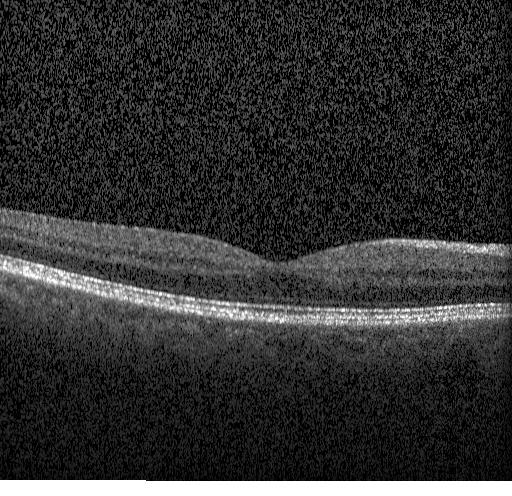

SD-OCT, retinal OCT cross-section, fovea-centered — OCT finding: no evidence of CNV, DME, or drusen.